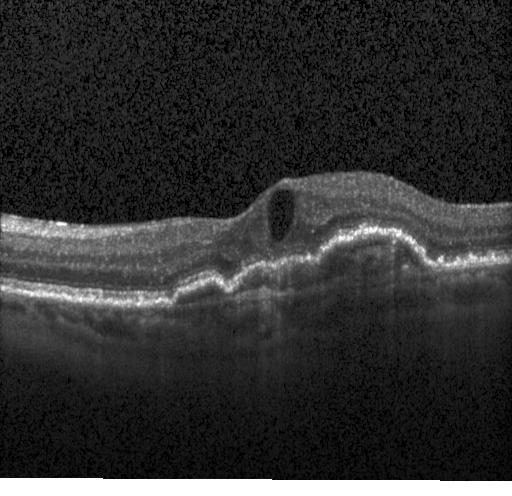 OCT B-scan.
Impression: a choroidal neovascular membrane.